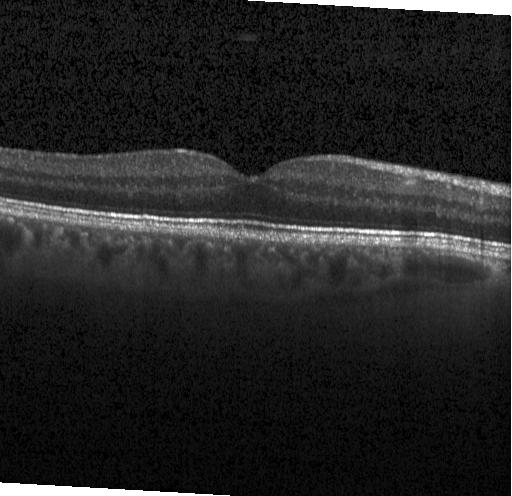 OCT scan showing no CNV, DME, or drusen.